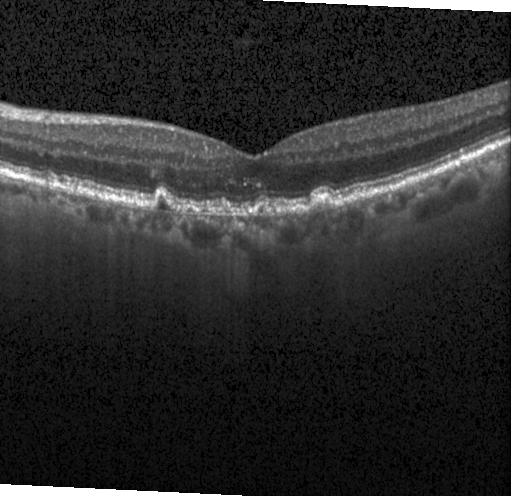
OCT finding: a choroidal neovascular membrane.